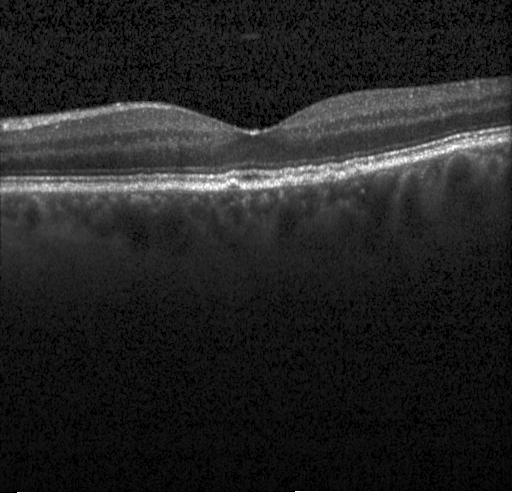

Dx: multiple drusen.